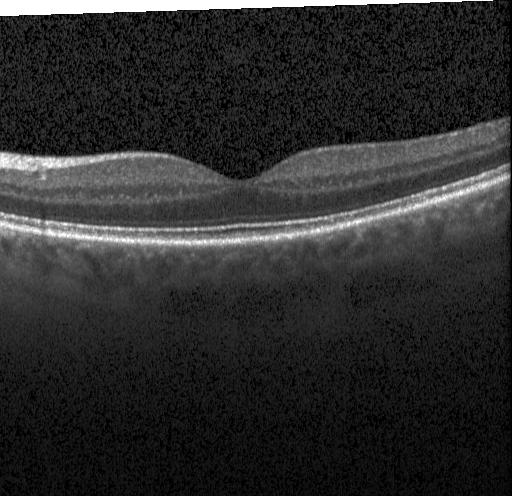
Dx: no evidence of choroidal neovascularization, diabetic macular edema, or drusen.